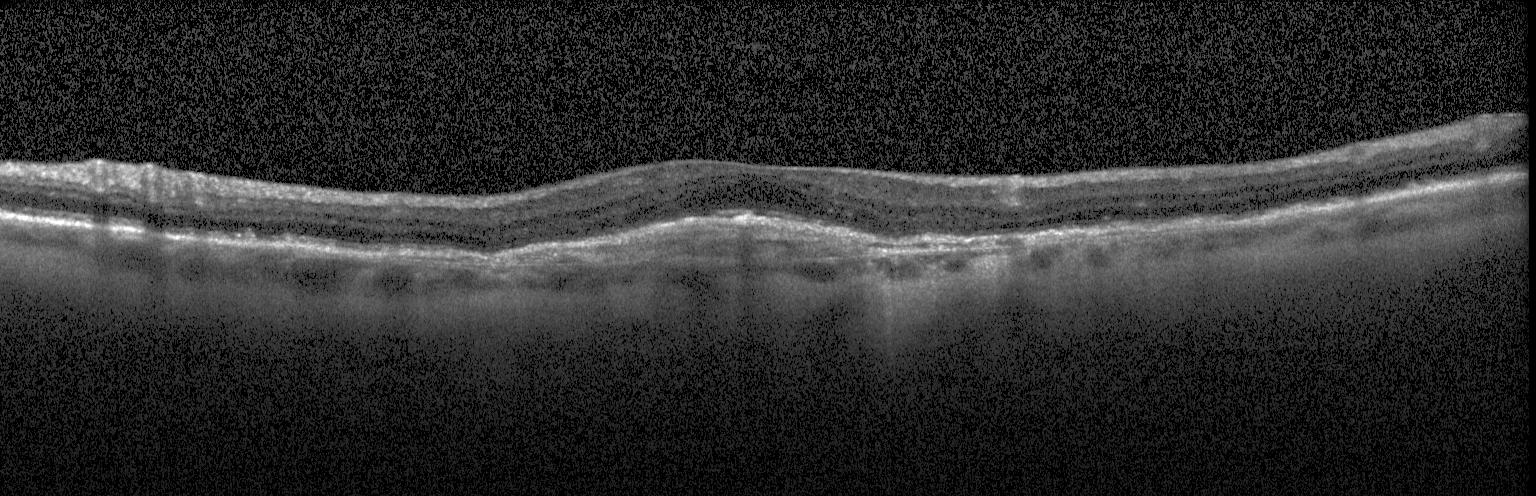

Retinal OCT cross-section showing CNV.